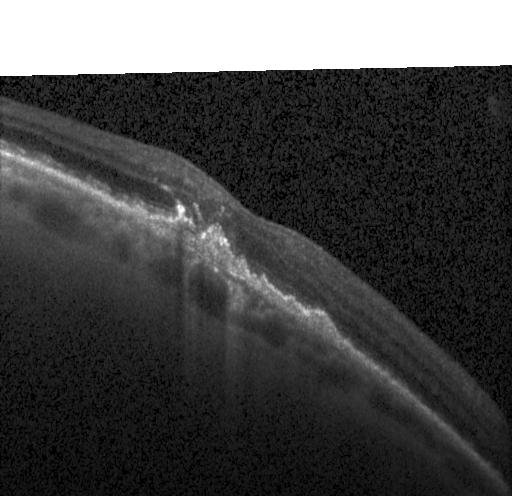 OCT line scan, horizontal scan through the fovea — CNV.